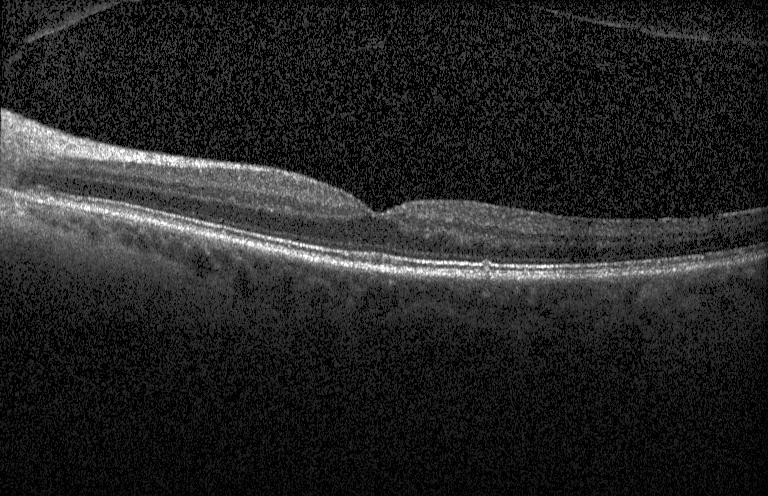
Impression: drusen.